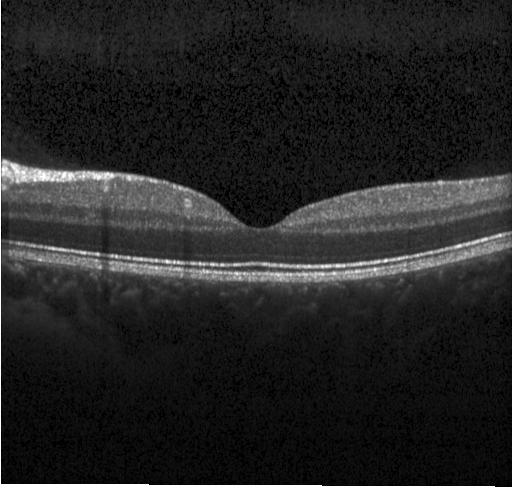
Retinal OCT B-scan. Acquired on a Heidelberg Spectralis.
Impression: neither choroidal neovascularization, diabetic macular edema, nor drusen.